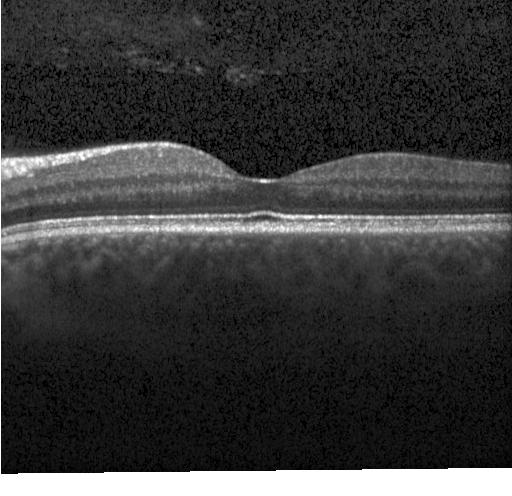 Optical coherence tomography scan · instrument: Heidelberg Spectralis · spectral-domain OCT · macular scan. Dx: no CNV, DME, or drusen.